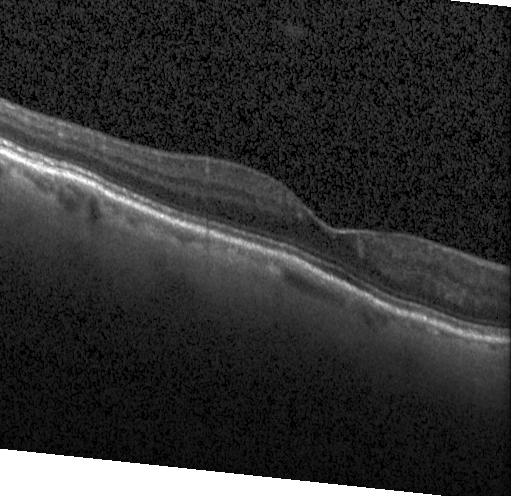 Finding: no choroidal neovascularization, no diabetic macular edema, and no drusen.